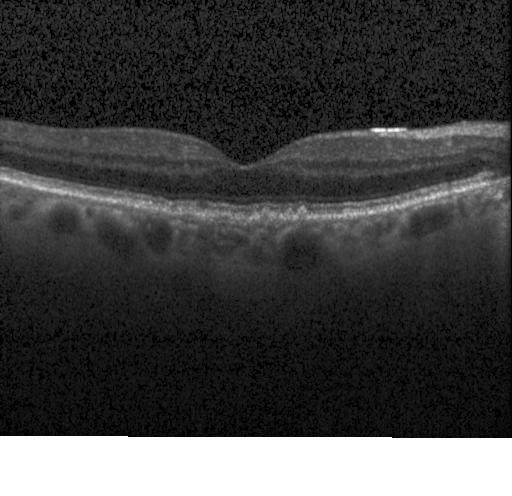 Spectral-domain OCT B-scan: drusen.